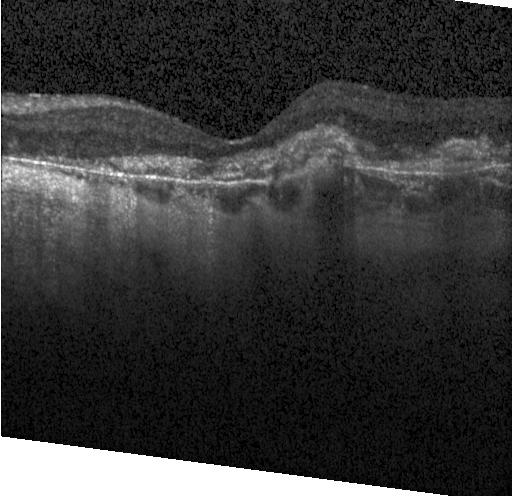 Retinal OCT cross-section
Impression: a choroidal neovascular membrane.